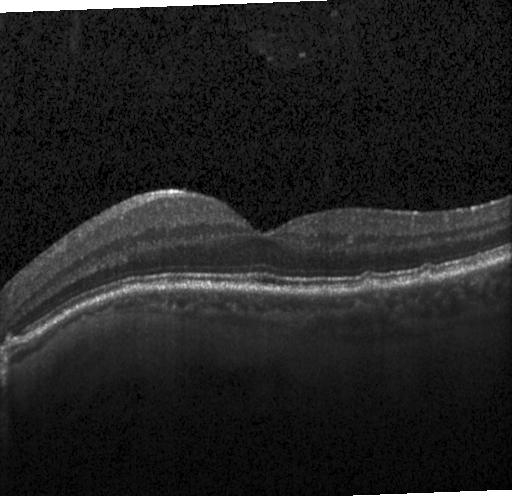 Spectral-domain OCT, optical coherence tomography B-scan, fovea-centered, instrument: Heidelberg Spectralis.
The scan shows sub-RPE drusenoid deposits.